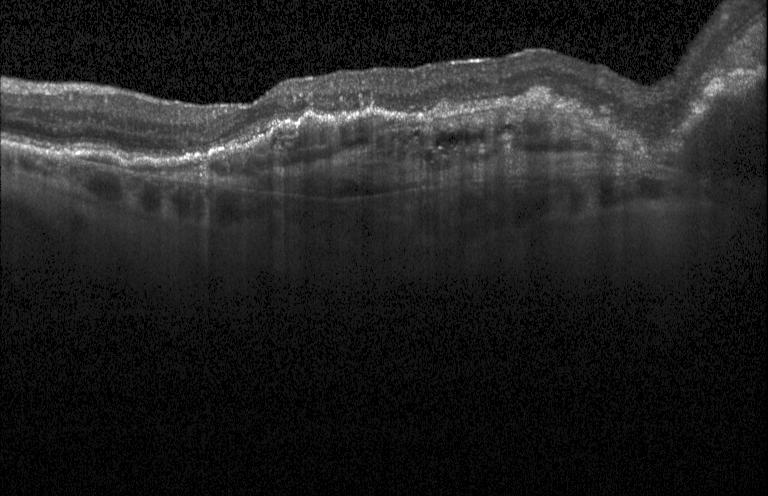

Heidelberg Spectralis. Retinal OCT cross-section. Spectral-domain optical coherence tomography
Diagnosis: a choroidal neovascular membrane.